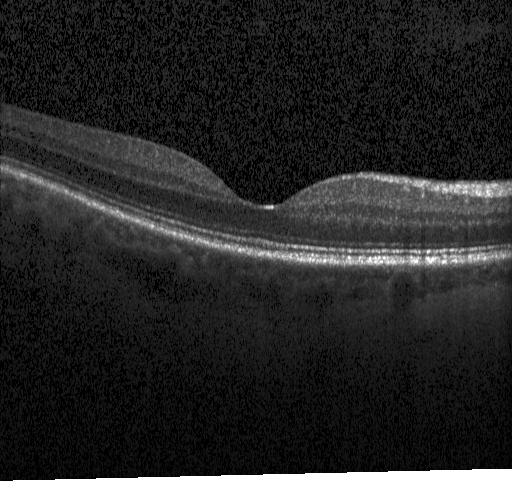 Optical coherence tomography scan — Finding: no choroidal neovascularization, no diabetic macular edema, and no drusen.